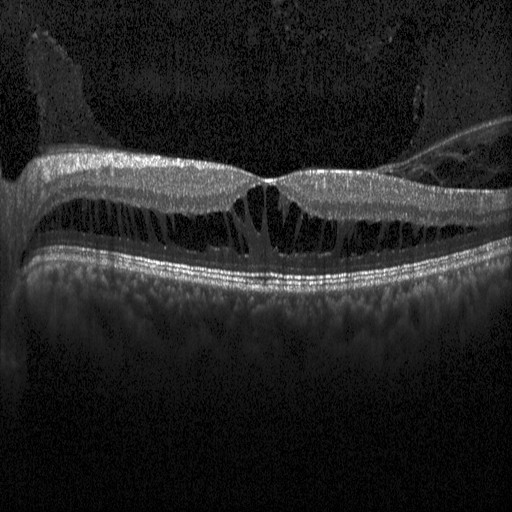

Optical coherence tomography B-scan, macular scan — Finding: DME.